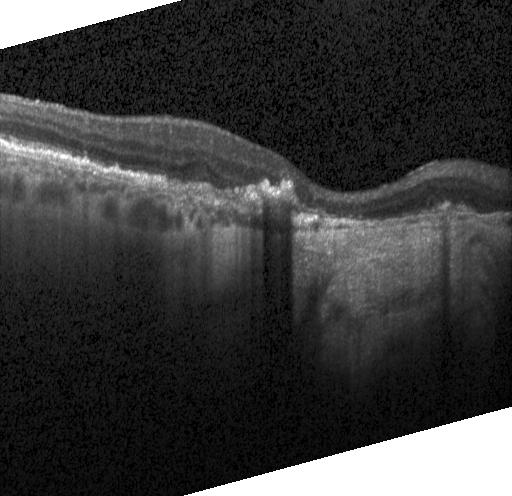

Macular OCT demonstrating a choroidal neovascular membrane.